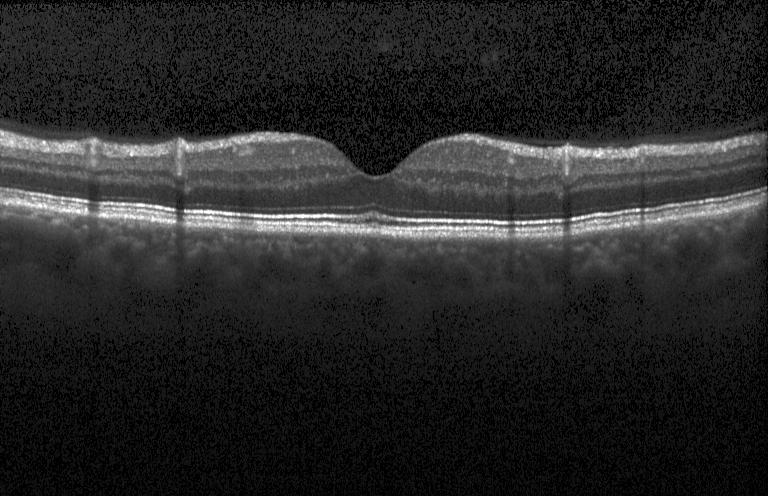 Centered on the fovea. SD-OCT. OCT line scan. Instrument: Heidelberg Spectralis.
Finding: no choroidal neovascularization, diabetic macular edema, or drusen.